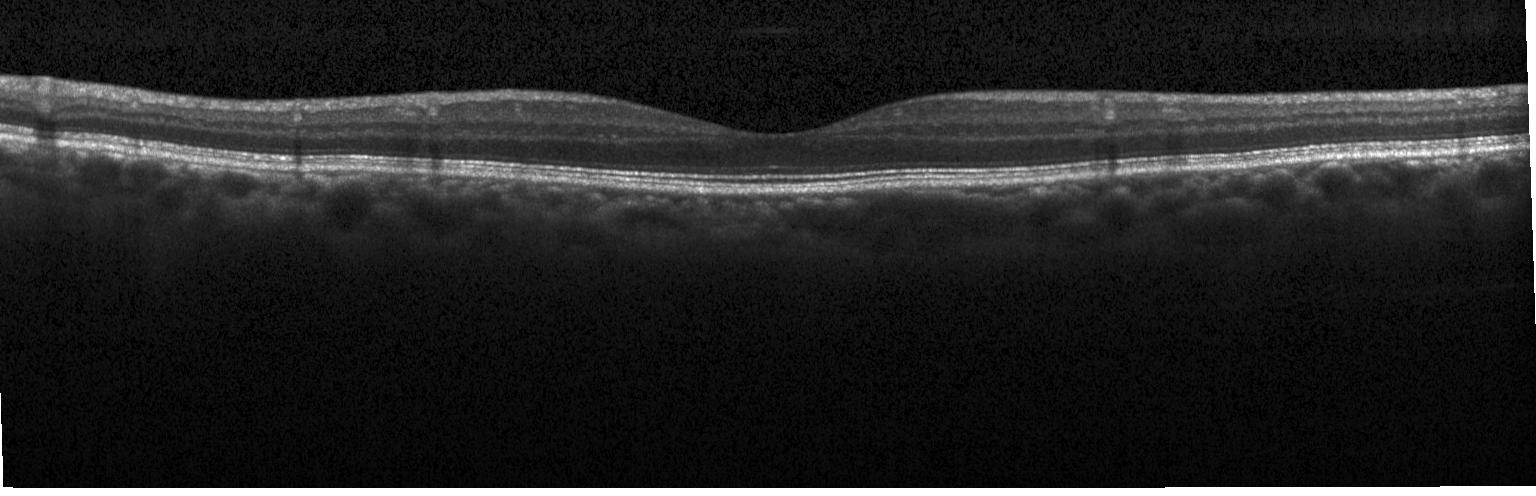 Acquired on a Heidelberg Spectralis; optical coherence tomography scan; centered on the fovea.
Finding: neither choroidal neovascularization, diabetic macular edema, nor drusen.